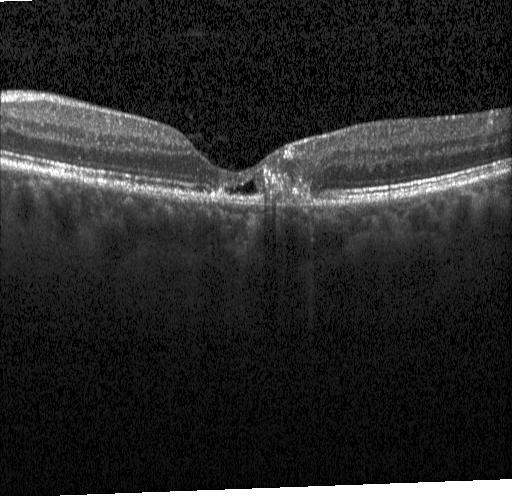 Macular OCT: CNV.